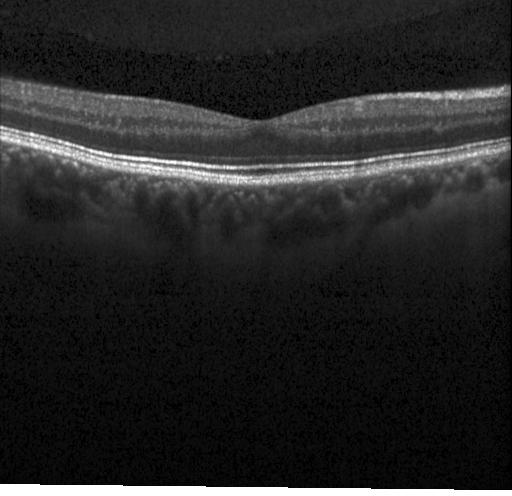
Retinal OCT cross-section
Finding: no evidence of choroidal neovascularization, diabetic macular edema, or drusen.